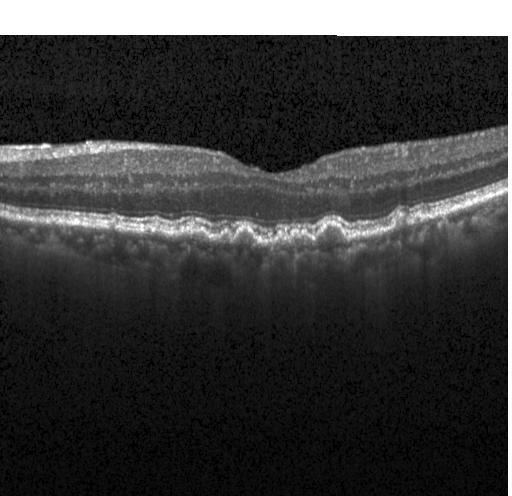
Optical coherence tomography scan; through the macula; spectral-domain OCT — Finding: multiple drusen.